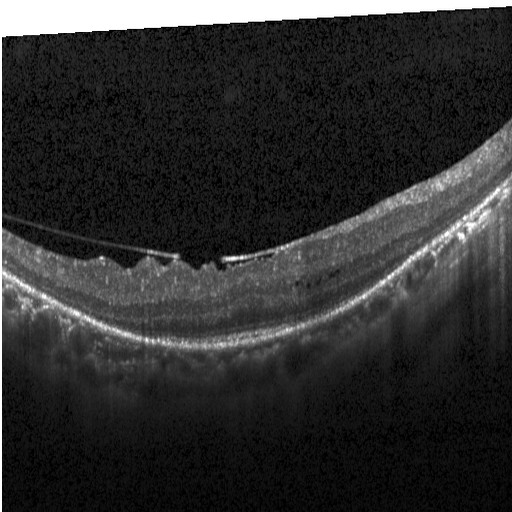

Centered on the fovea, SD-OCT, retinal OCT cross-section, Heidelberg Spectralis OCT system. Impression: diabetic macular edema.